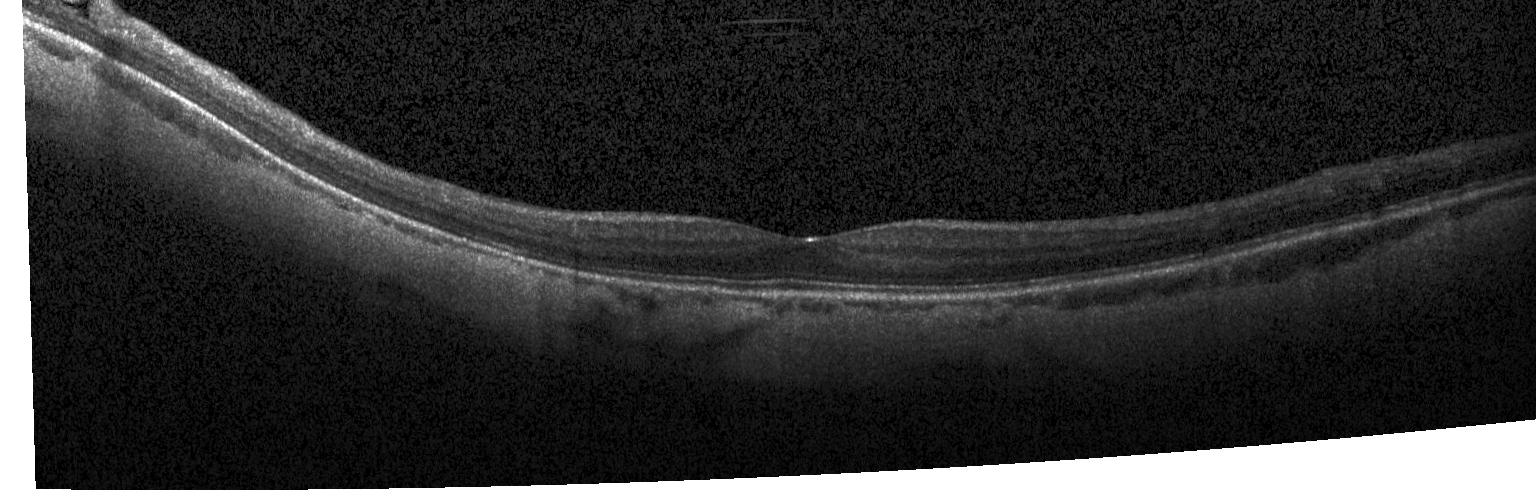 OCT line scan, through the macula. Diagnosis: neither CNV, DME, nor drusen.